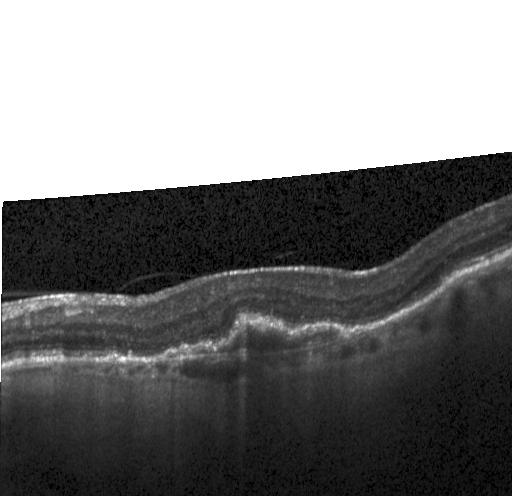
Impression: a choroidal neovascular membrane.